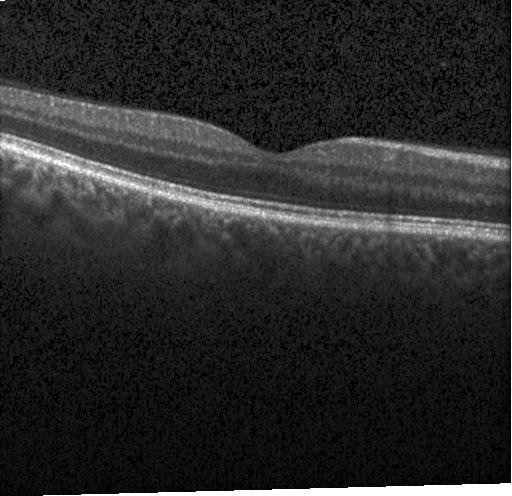 Spectral-domain optical coherence tomography, optical coherence tomography B-scan.
Dx: no evidence of choroidal neovascularization, diabetic macular edema, or drusen.